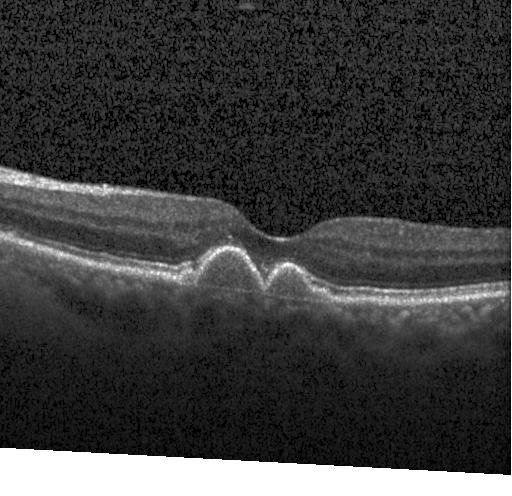 Drusen.